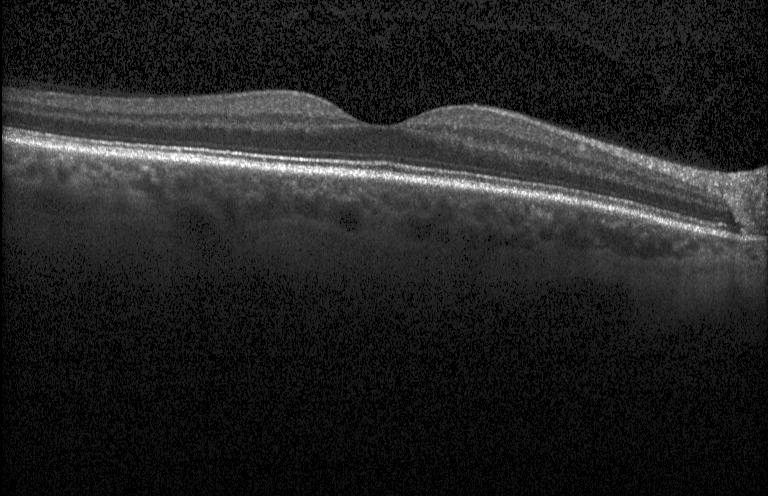
Heidelberg Spectralis OCT system. Retinal OCT B-scan. Fovea-centered. Spectral-domain optical coherence tomography. Diagnosis: no choroidal neovascularization, diabetic macular edema, or drusen.